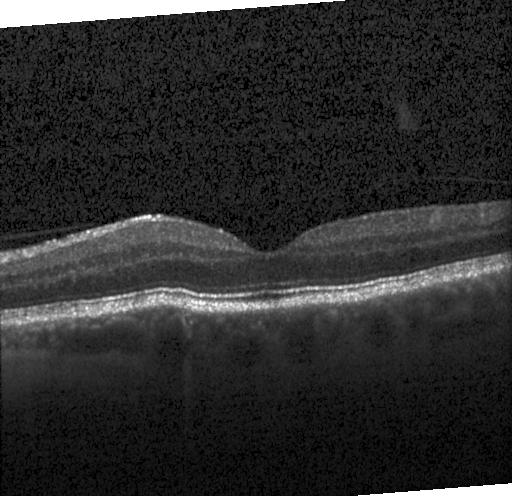

Horizontal scan through the fovea · OCT B-scan. Diagnosis: no choroidal neovascularization, diabetic macular edema, or drusen.